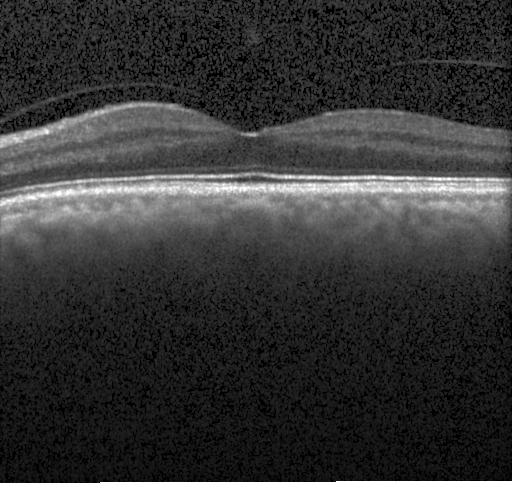

Retinal OCT B-scan · SD-OCT · acquired on a Heidelberg Spectralis · fovea-centered.
No choroidal neovascularization, diabetic macular edema, or drusen.